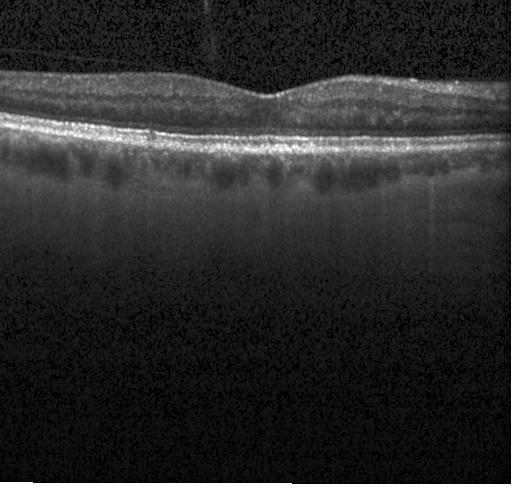 Heidelberg Spectralis, OCT B-scan, through the macula, spectral-domain OCT.
No evidence of choroidal neovascularization, diabetic macular edema, or drusen.